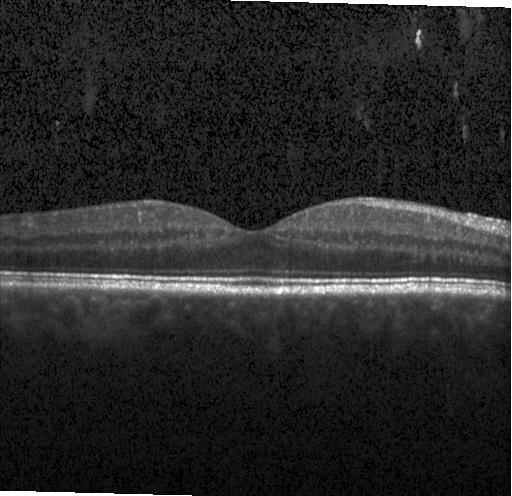

Spectral-domain optical coherence tomography, Heidelberg Spectralis, retinal OCT B-scan. Assessment: no choroidal neovascularization, diabetic macular edema, or drusen.